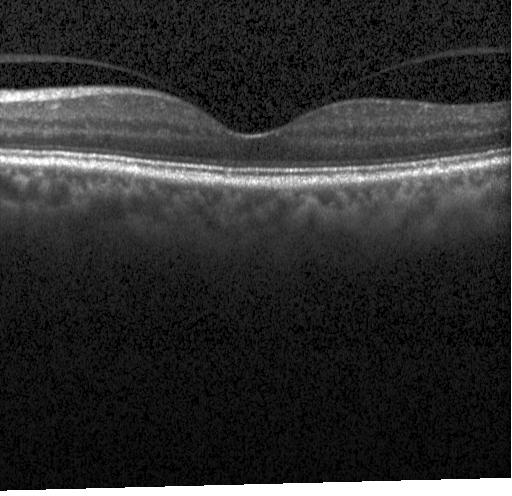

Spectral-domain OCT B-scan: no choroidal neovascularization, diabetic macular edema, or drusen.